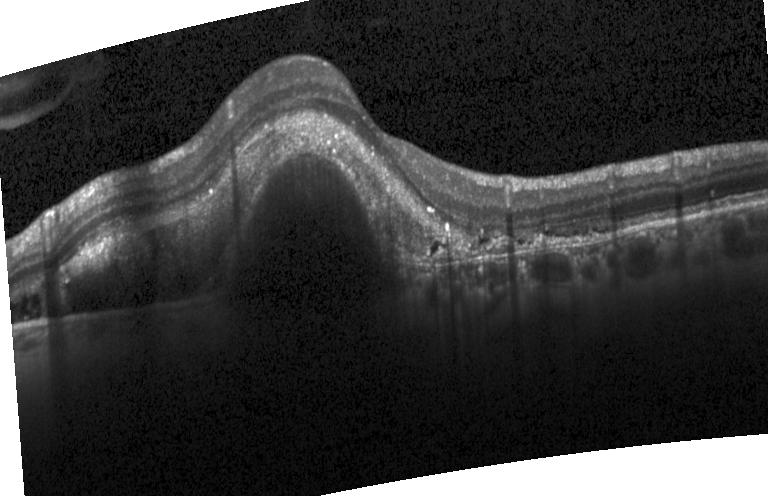

OCT B-scan. Diagnosis: CNV.